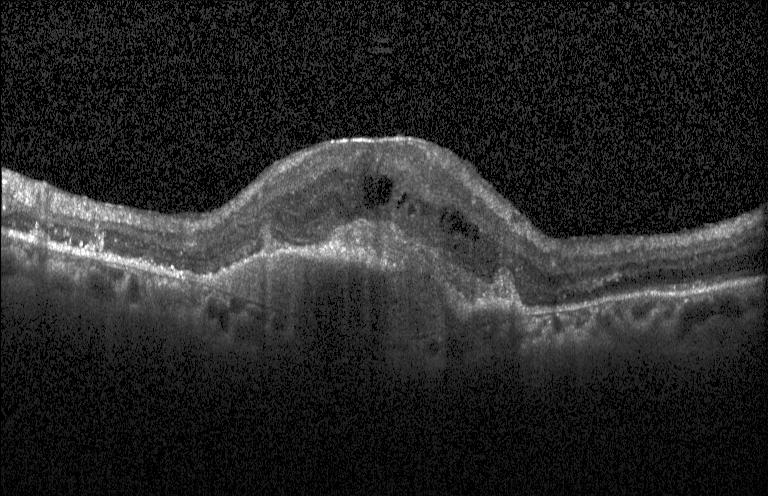 Impression: CNV.